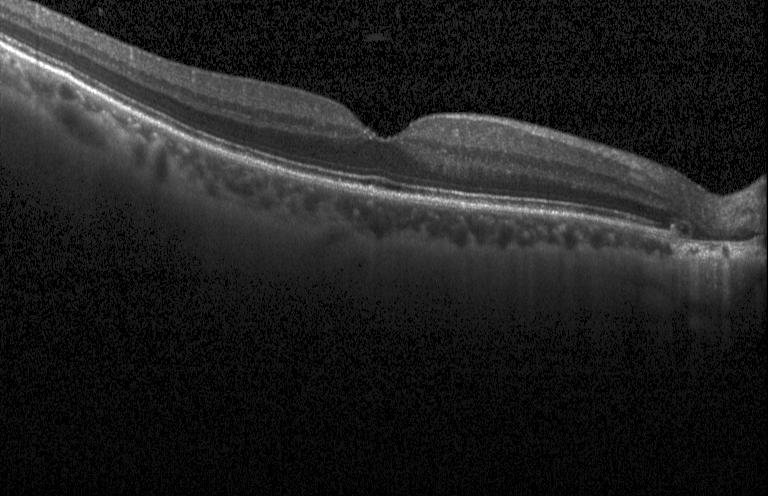

Heidelberg Spectralis. Centered on the fovea. SD-OCT. Retinal OCT B-scan
This B-scan demonstrates no evidence of choroidal neovascularization, diabetic macular edema, or drusen.